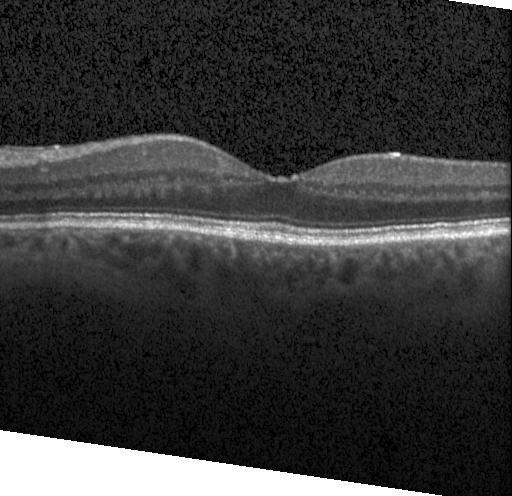

Retinal OCT cross-section
This B-scan demonstrates neither CNV, DME, nor drusen.